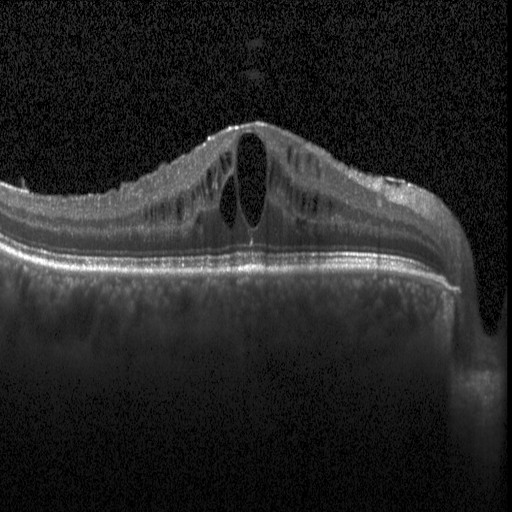

Diagnosis: diabetic macular edema.